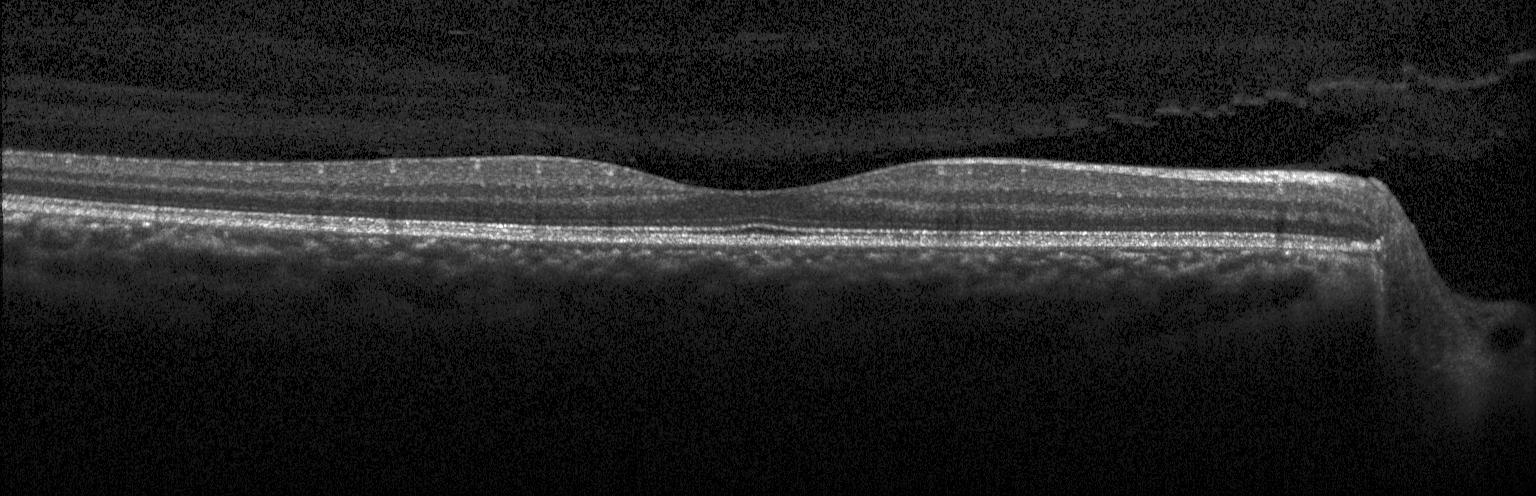 Spectral-domain optical coherence tomography · fovea-centered · retinal OCT cross-section · Heidelberg Spectralis OCT system. OCT finding: no CNV, DME, or drusen.